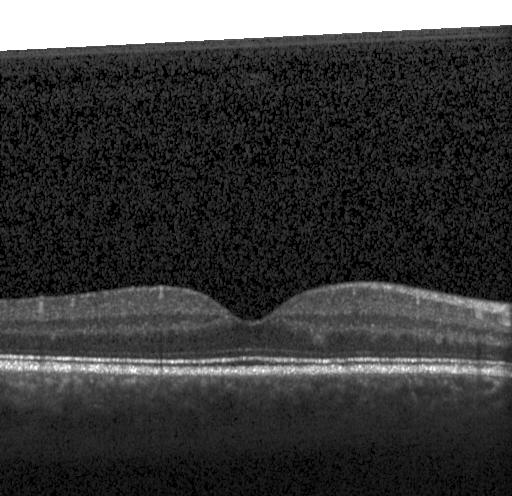
No choroidal neovascularization, no diabetic macular edema, and no drusen.